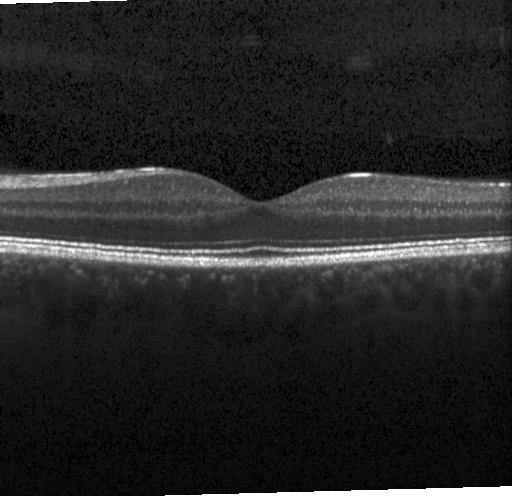

OCT B-scan — Assessment: no evidence of choroidal neovascularization, diabetic macular edema, or drusen.